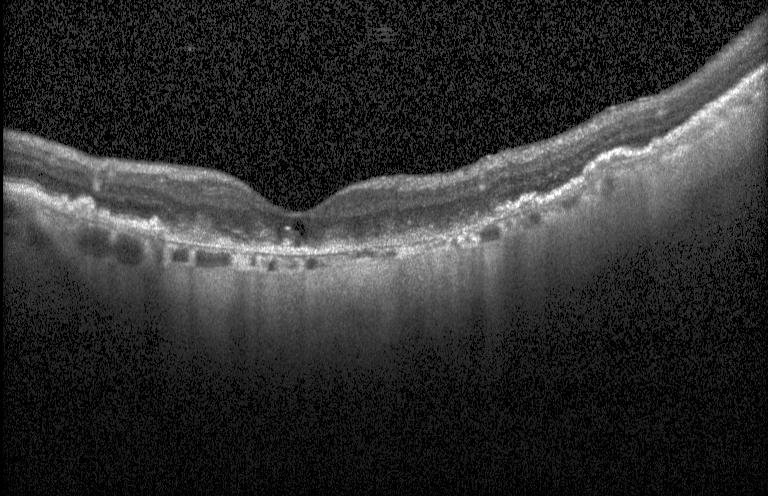 OCT B-scan — Impression: a choroidal neovascular membrane.